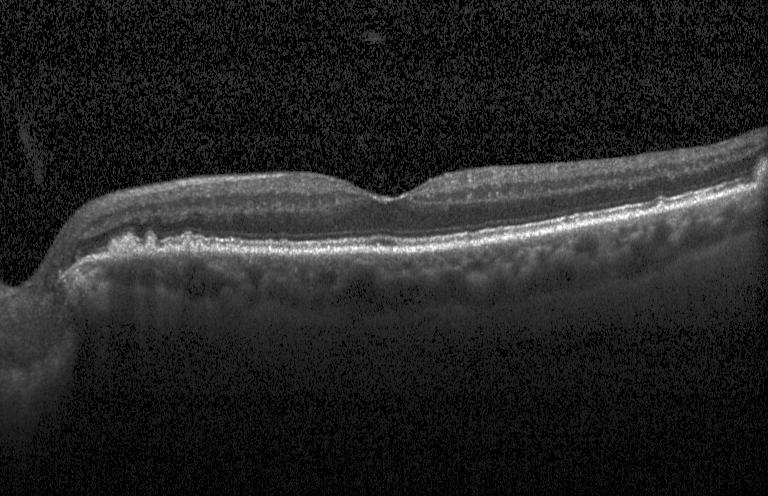
SD-OCT · retinal OCT cross-section · through the macula.
Diagnosis: multiple drusen.